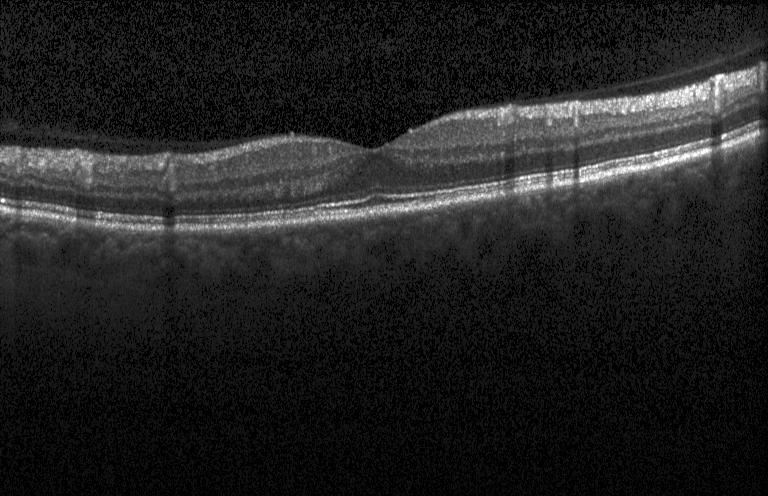 Finding: no choroidal neovascularization, no diabetic macular edema, and no drusen.